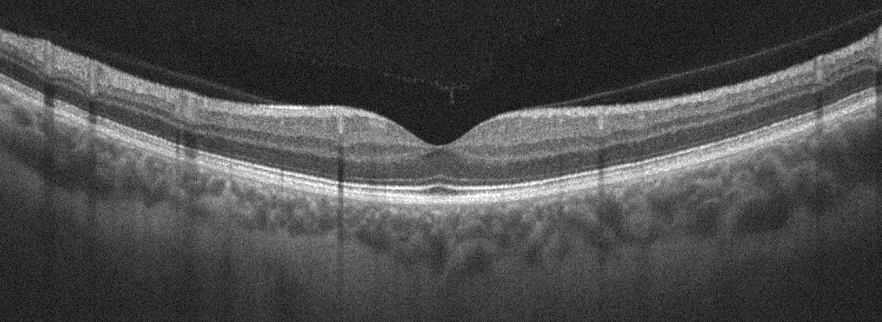 Optical coherence tomography B-scan. Diagnosis: no evidence of AMD, DME, ERM, RAO, RVO, or VID.